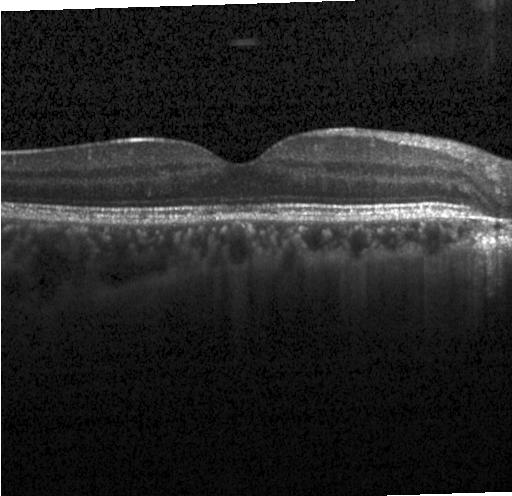

Centered on the fovea · optical coherence tomography scan · Heidelberg Spectralis. No evidence of CNV, DME, or drusen.